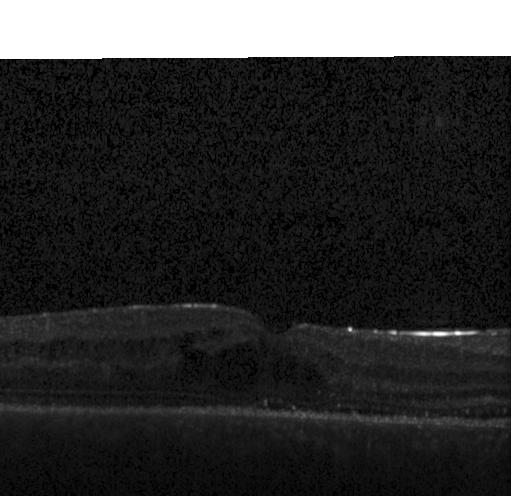
This B-scan demonstrates diabetic macular edema.